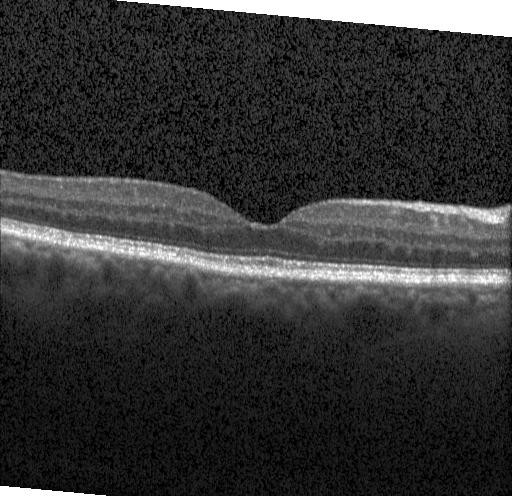
Spectral-domain OCT B-scan: no CNV, DME, or drusen.